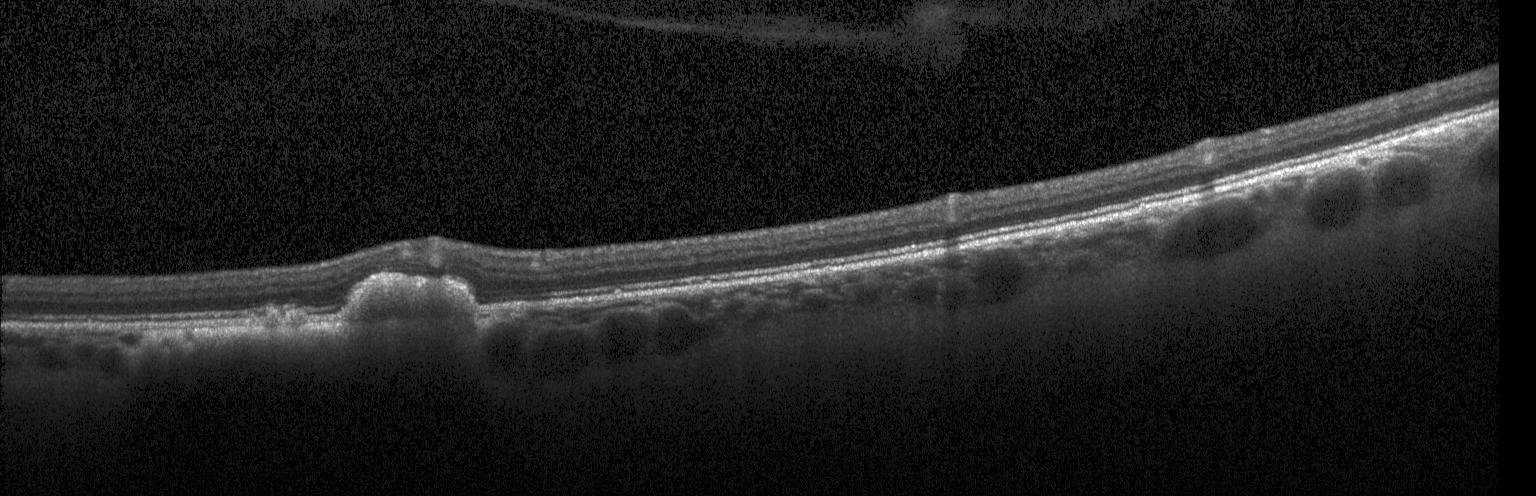 Retinal OCT B-scan
Diagnosis: a choroidal neovascular membrane.